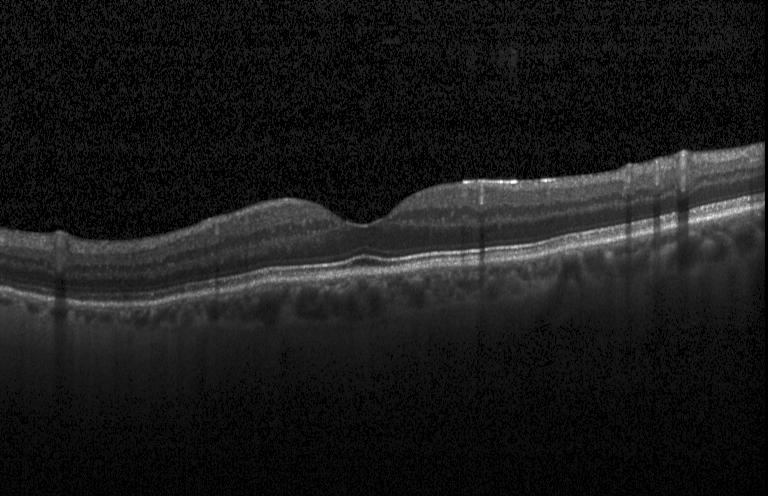
This B-scan demonstrates no choroidal neovascularization, no diabetic macular edema, and no drusen.